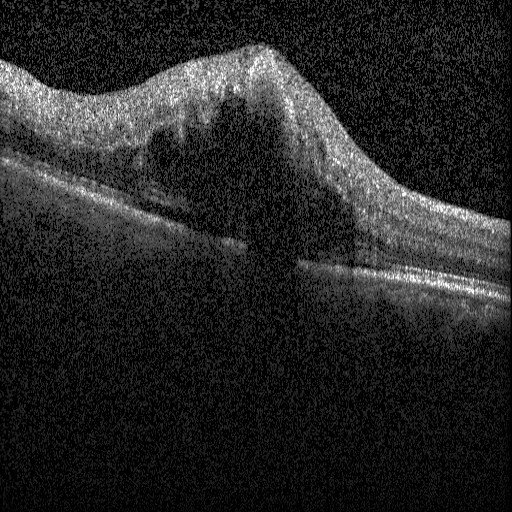

Heidelberg Spectralis OCT system; optical coherence tomography scan
The scan shows diabetic macular edema (DME).